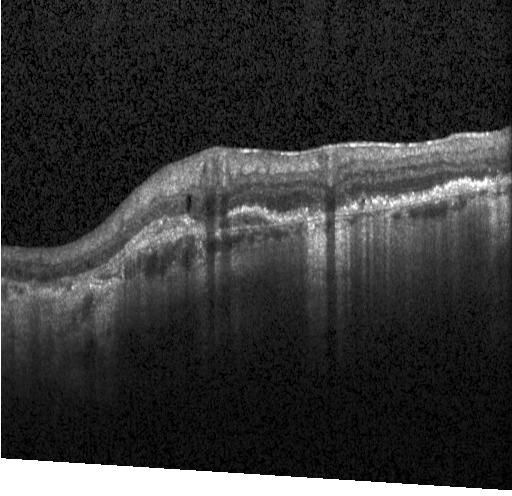
SD-OCT, optical coherence tomography scan, acquired on a Heidelberg Spectralis, fovea-centered. A choroidal neovascular membrane.